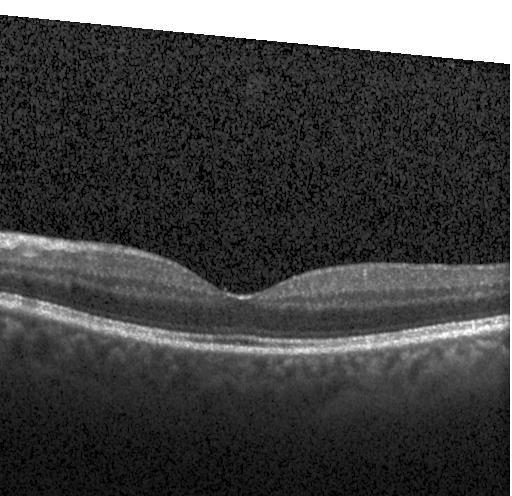 This B-scan demonstrates no CNV, DME, or drusen.